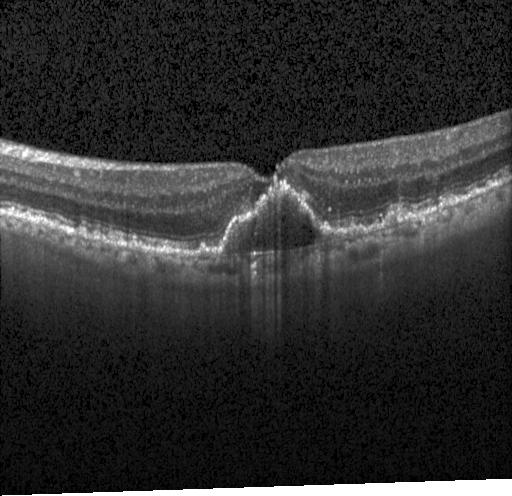 Assessment: choroidal neovascularization.